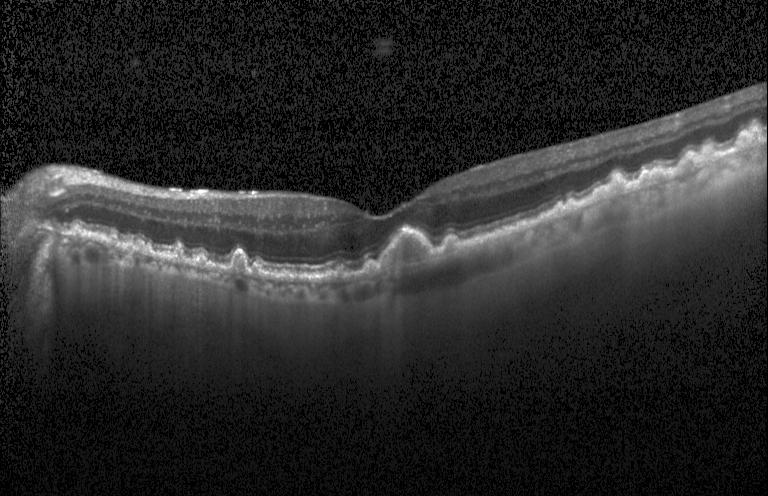
Dx: sub-RPE drusenoid deposits.